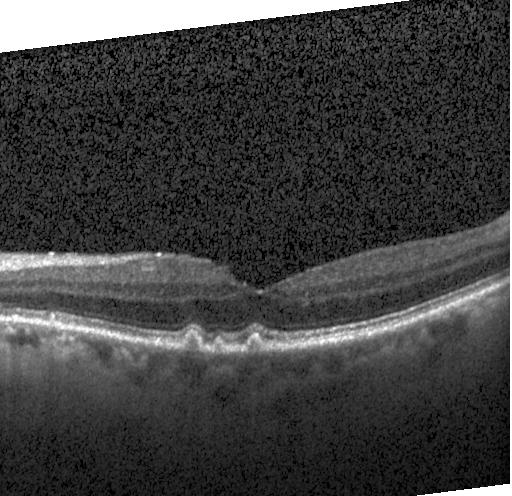

OCT B-scan showing multiple drusen.